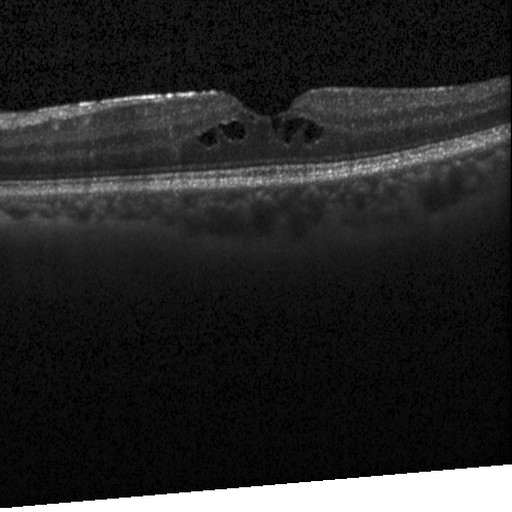

Finding: diabetic macular edema (DME).